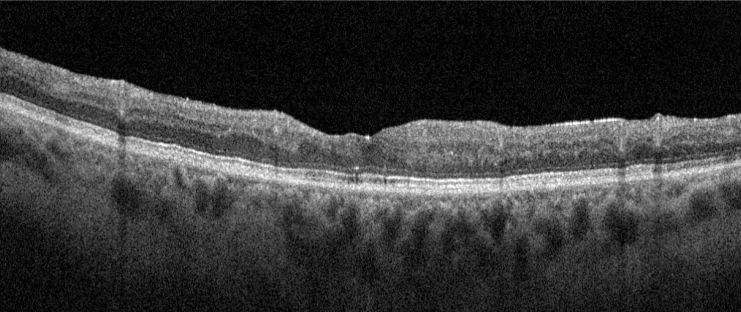 OCT B-scan.
Macular OCT: diabetic macular edema.